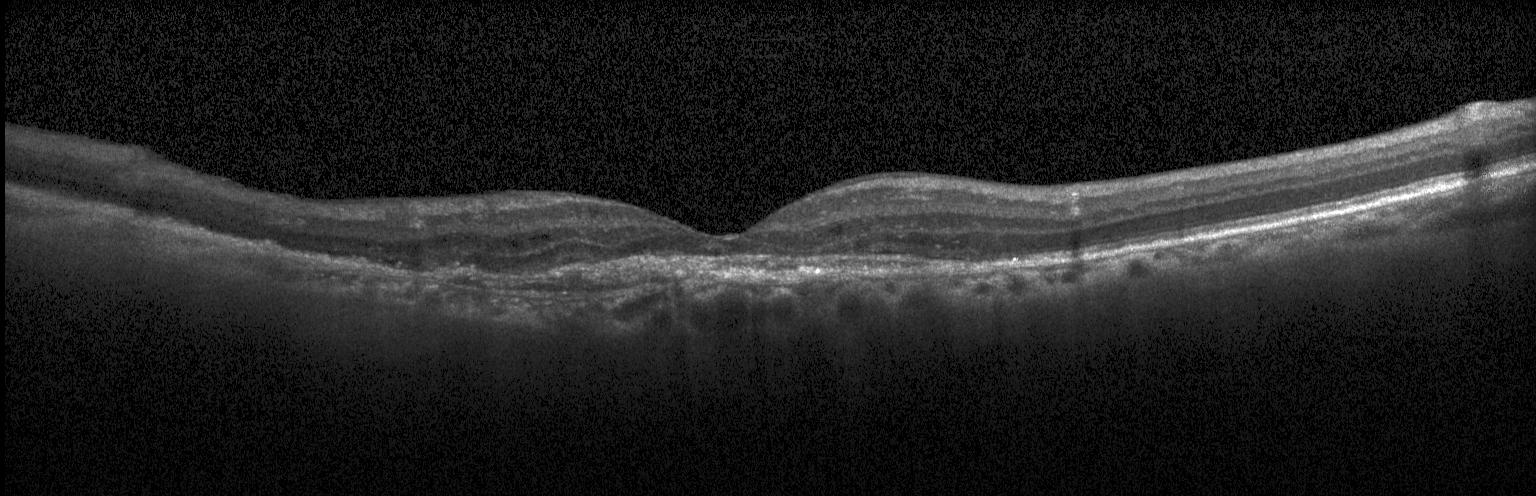 Retinal OCT cross-section — A choroidal neovascular membrane.